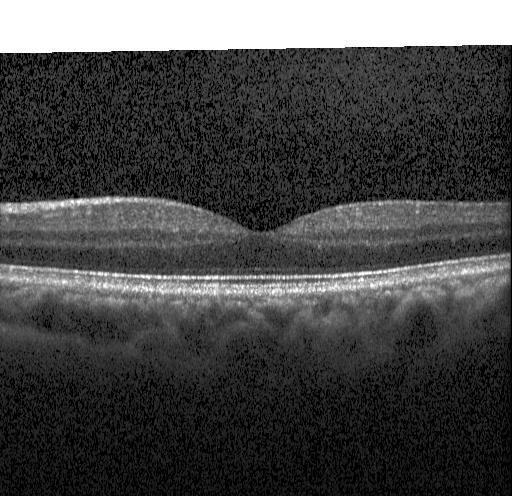
Optical coherence tomography B-scan
Diagnosis: no evidence of choroidal neovascularization, diabetic macular edema, or drusen.